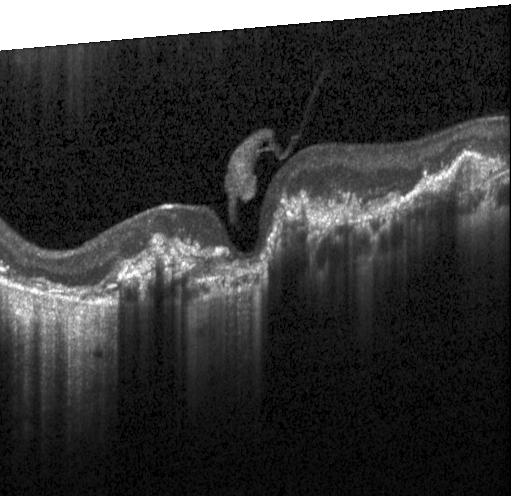 Optical coherence tomography B-scan. OCT finding: CNV.